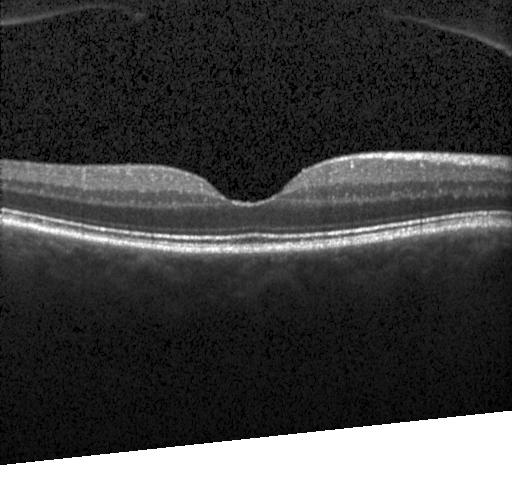 Dx: no evidence of choroidal neovascularization, diabetic macular edema, or drusen.